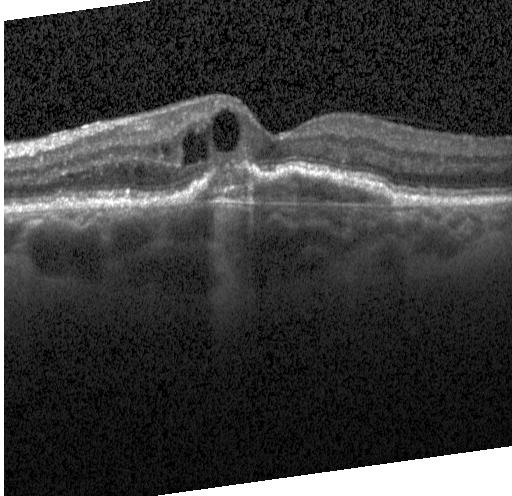

Fovea-centered · SD-OCT · retinal OCT B-scan
Finding: a choroidal neovascular membrane.